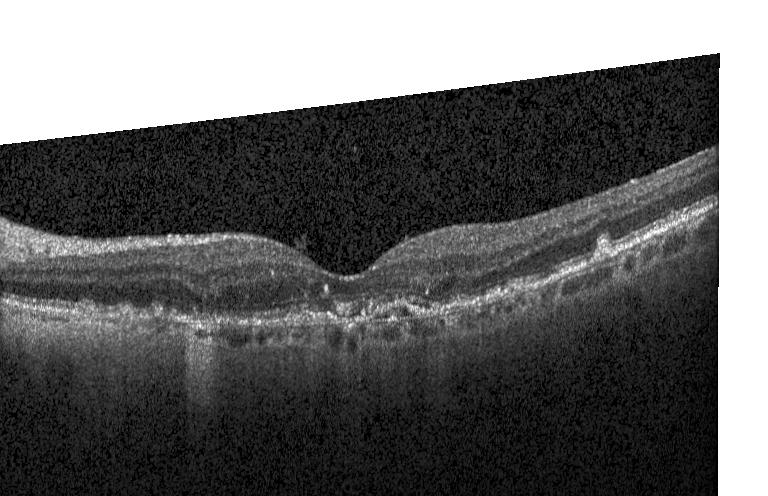 Horizontal scan through the fovea, retinal OCT B-scan
This B-scan demonstrates choroidal neovascularization (CNV).